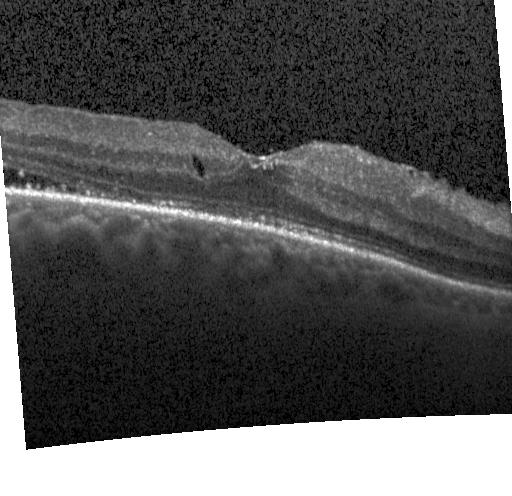
Impression: DME.